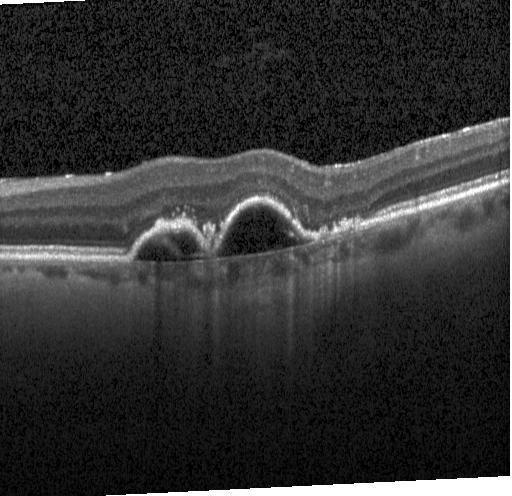
OCT scan showing a choroidal neovascular membrane.